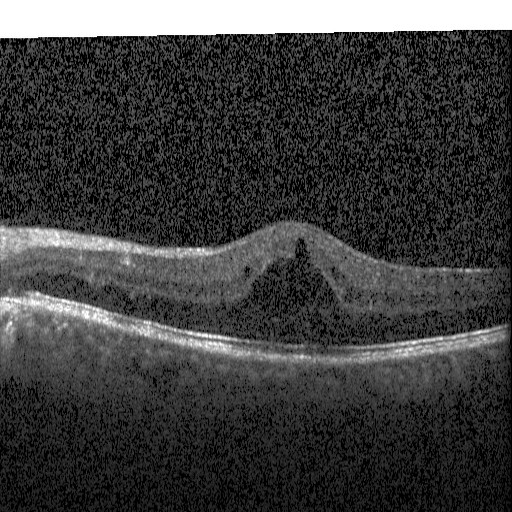
OCT line scan.
This B-scan demonstrates diabetic macular edema.